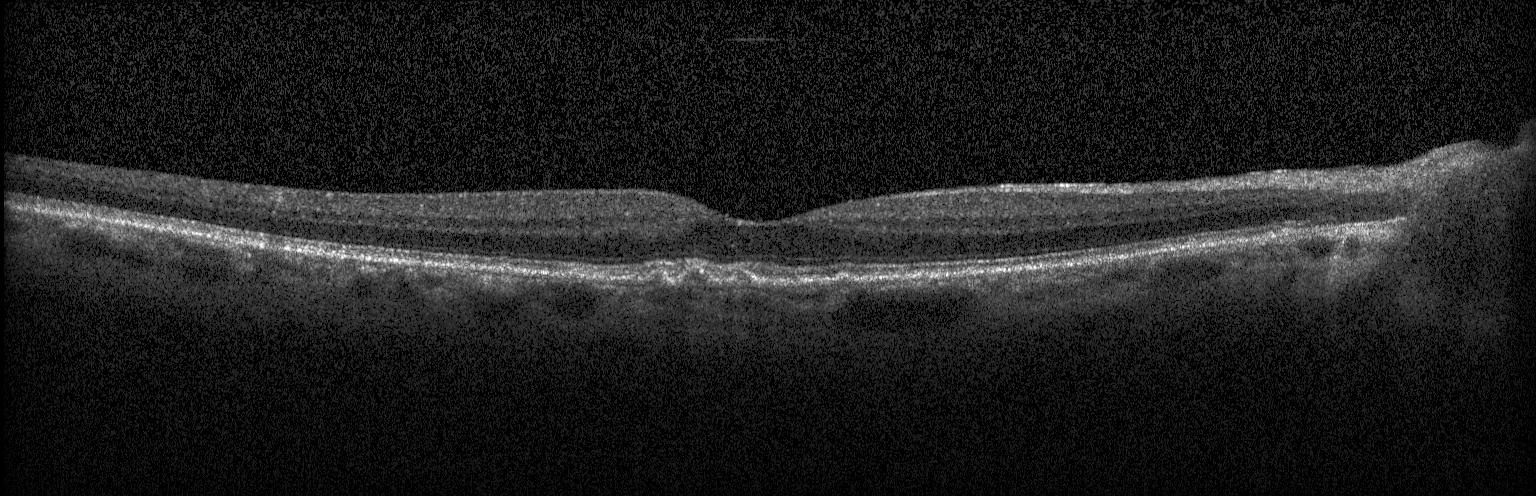
This B-scan demonstrates drusen.